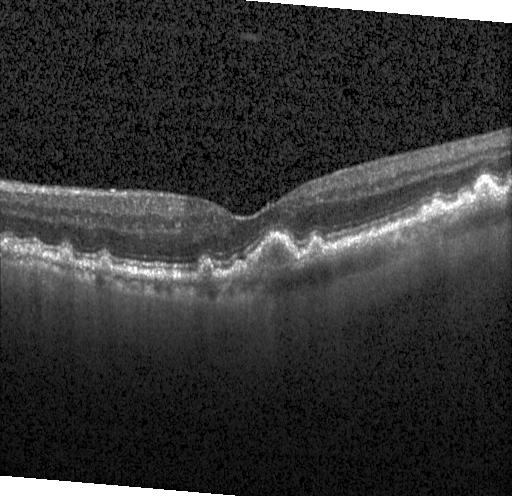

Sub-RPE drusenoid deposits.